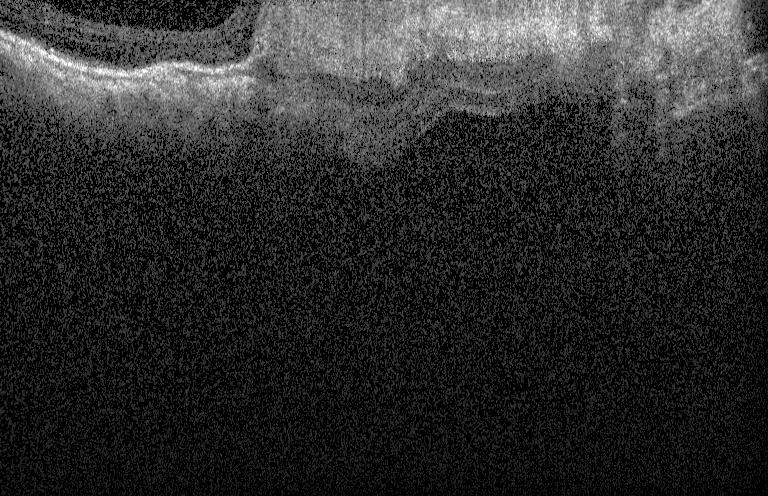
OCT finding: a choroidal neovascular membrane.